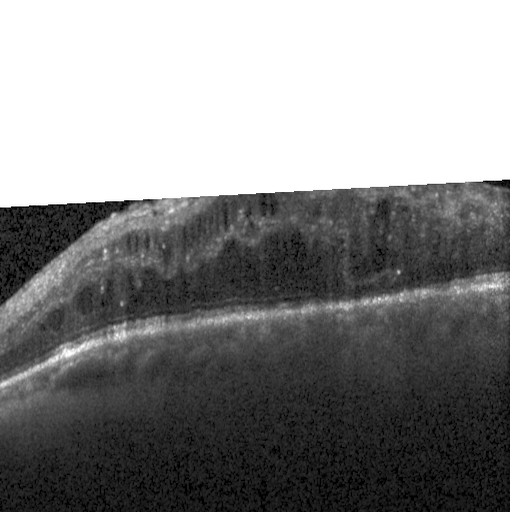

Impression: DME.